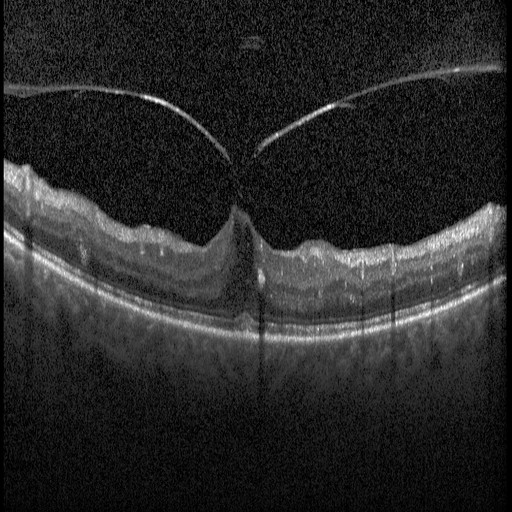
Impression: diabetic macular edema (DME).